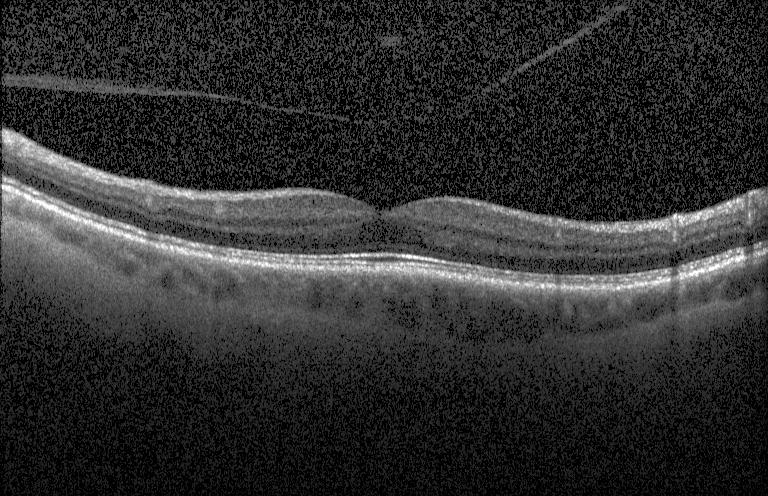

Optical coherence tomography B-scan; spectral-domain OCT; centered on the fovea; acquired on a Heidelberg Spectralis — This B-scan demonstrates neither choroidal neovascularization, diabetic macular edema, nor drusen.